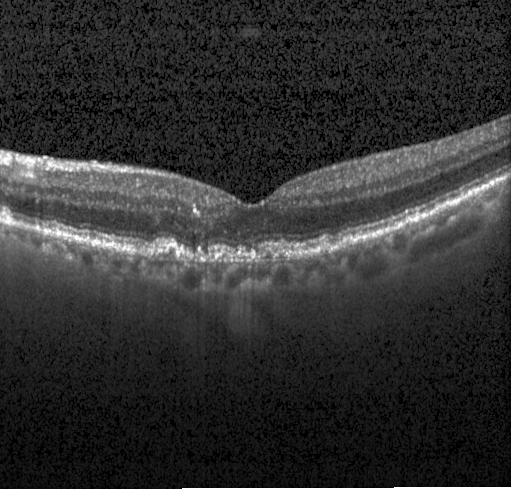
OCT B-scan.
Diagnosis: multiple drusen.